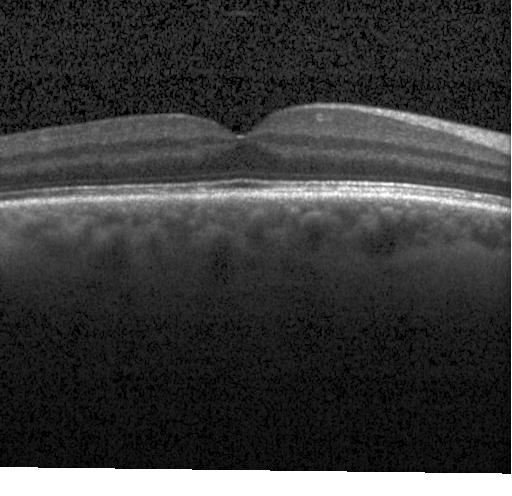

SD-OCT. OCT B-scan. Heidelberg Spectralis. Fovea-centered — Macular OCT: no choroidal neovascularization, diabetic macular edema, or drusen.